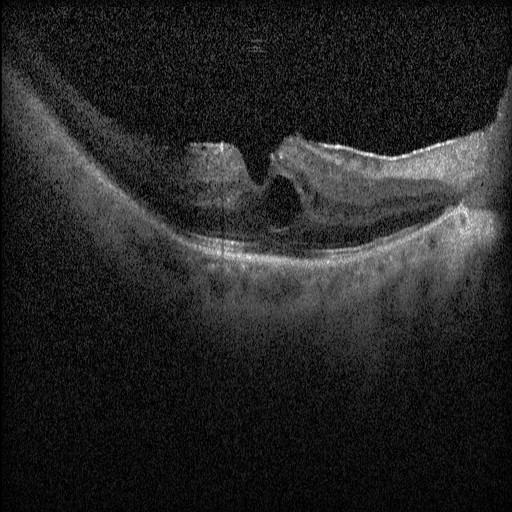 Heidelberg Spectralis OCT system; spectral-domain optical coherence tomography; horizontal scan through the fovea; retinal OCT cross-section — This B-scan demonstrates DME.